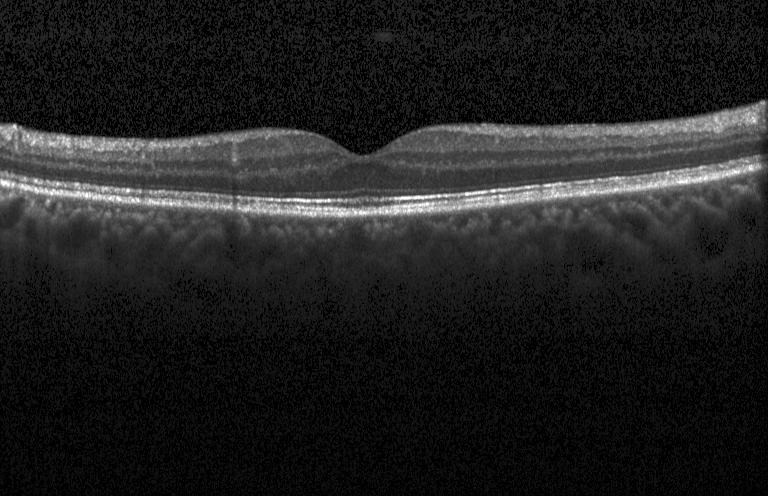 Optical coherence tomography scan; centered on the fovea. Dx: neither choroidal neovascularization, diabetic macular edema, nor drusen.